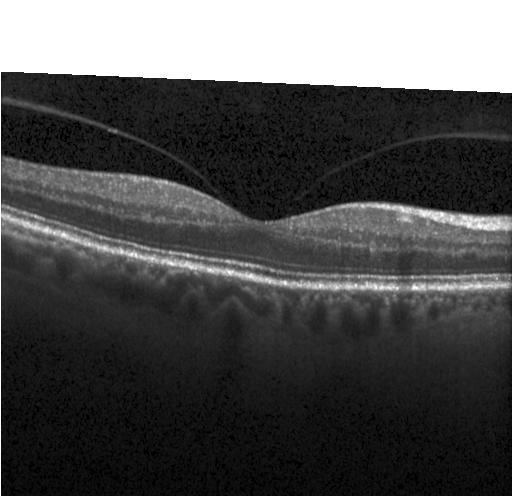 Finding: no evidence of choroidal neovascularization, diabetic macular edema, or drusen.